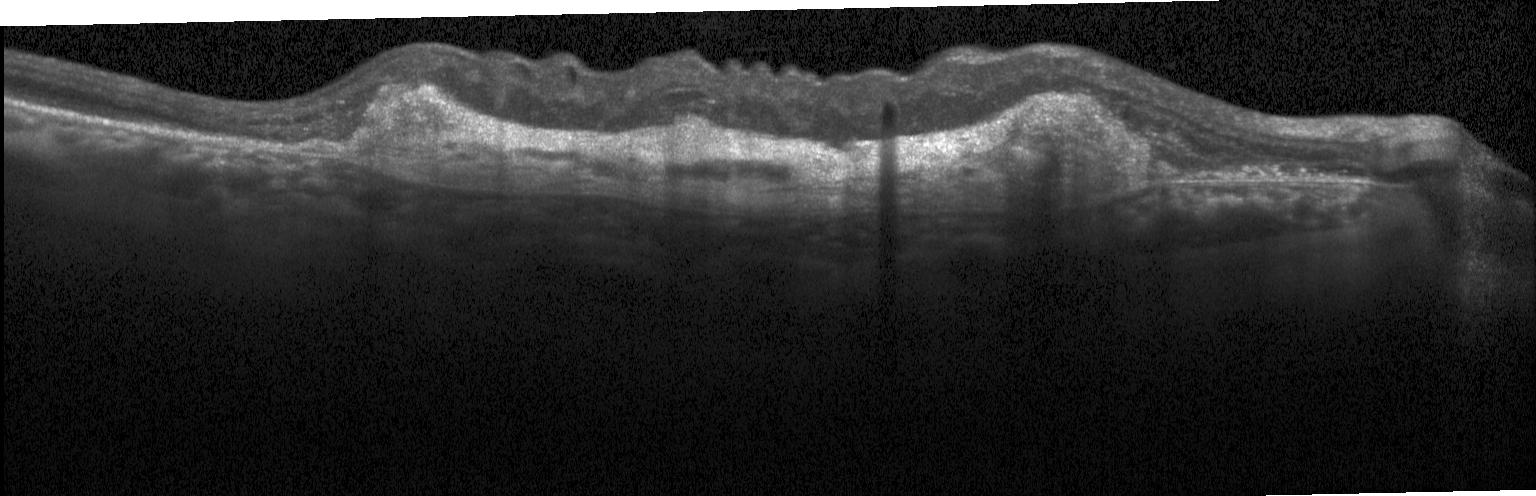
Heidelberg Spectralis OCT system; macular scan; optical coherence tomography scan; spectral-domain optical coherence tomography
Assessment: choroidal neovascularization (CNV).